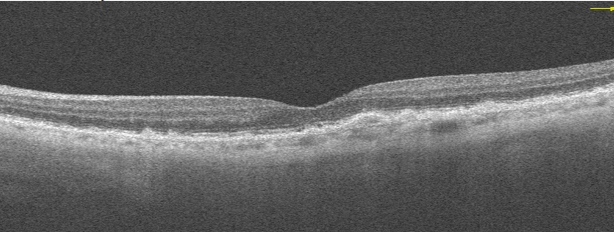

Diagnosis: age-related macular degeneration.